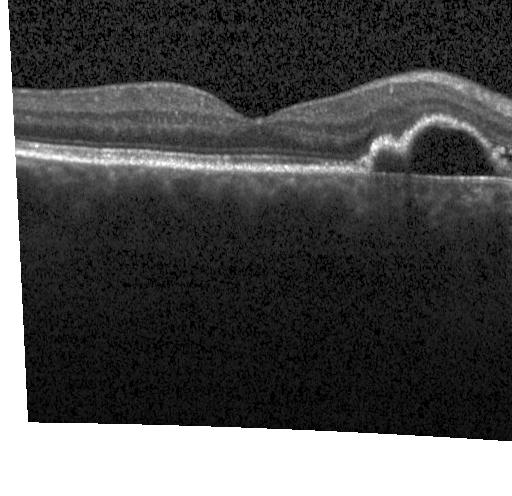

Through the macula. OCT line scan.
This B-scan demonstrates CNV.